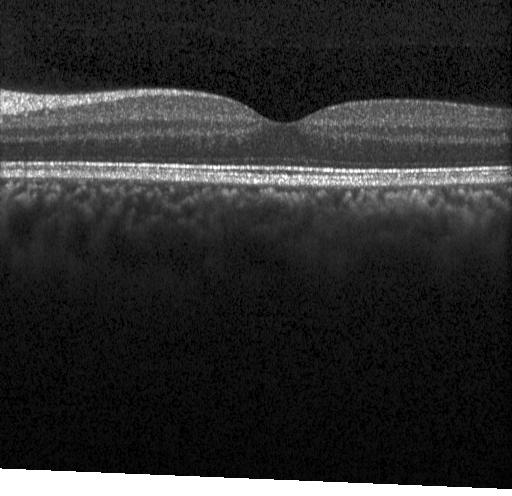 Assessment: no choroidal neovascularization, no diabetic macular edema, and no drusen.